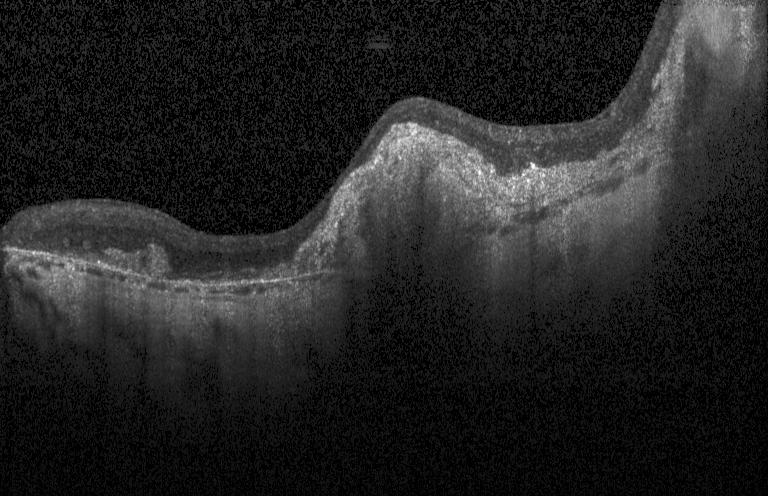

The scan shows a choroidal neovascular membrane.